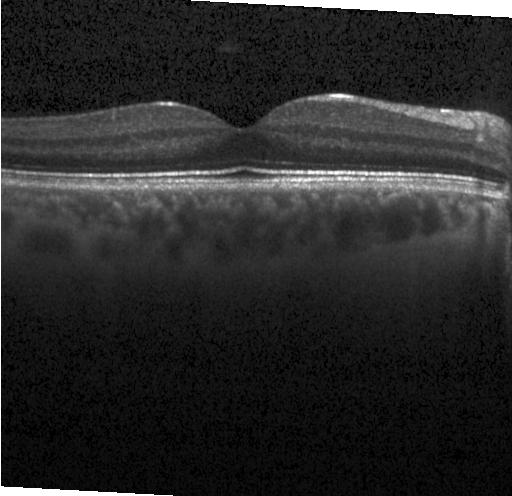
Retinal OCT B-scan. Finding: no choroidal neovascularization, diabetic macular edema, or drusen.